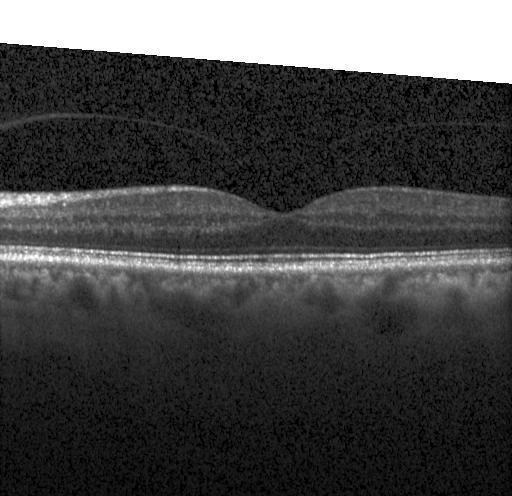
Retinal OCT cross-section · macular scan.
Diagnosis: no choroidal neovascularization, diabetic macular edema, or drusen.